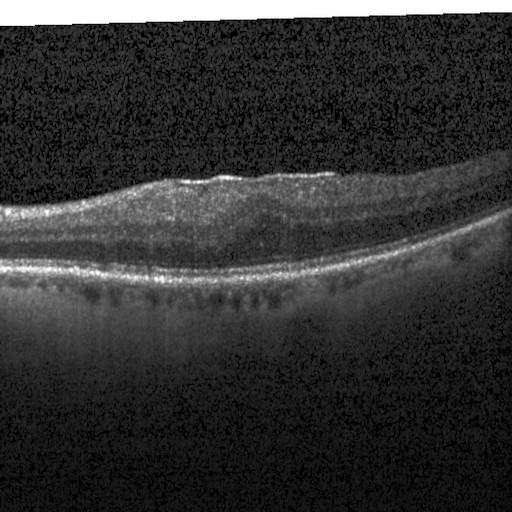 Heidelberg Spectralis OCT system · horizontal scan through the fovea · spectral-domain OCT · retinal OCT B-scan
Dx: diabetic macular edema.